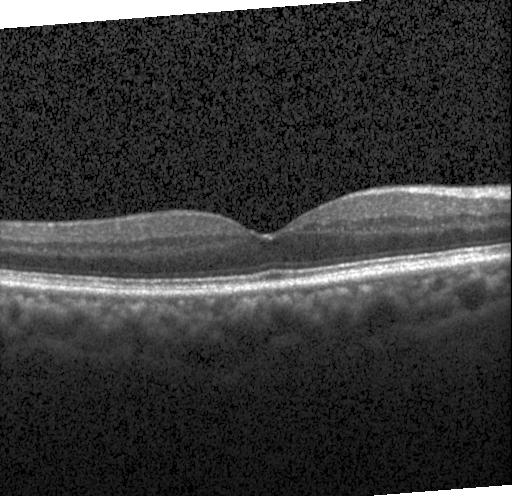

Centered on the fovea, acquired on a Heidelberg Spectralis, SD-OCT, retinal OCT cross-section — Finding: no choroidal neovascularization, no diabetic macular edema, and no drusen.